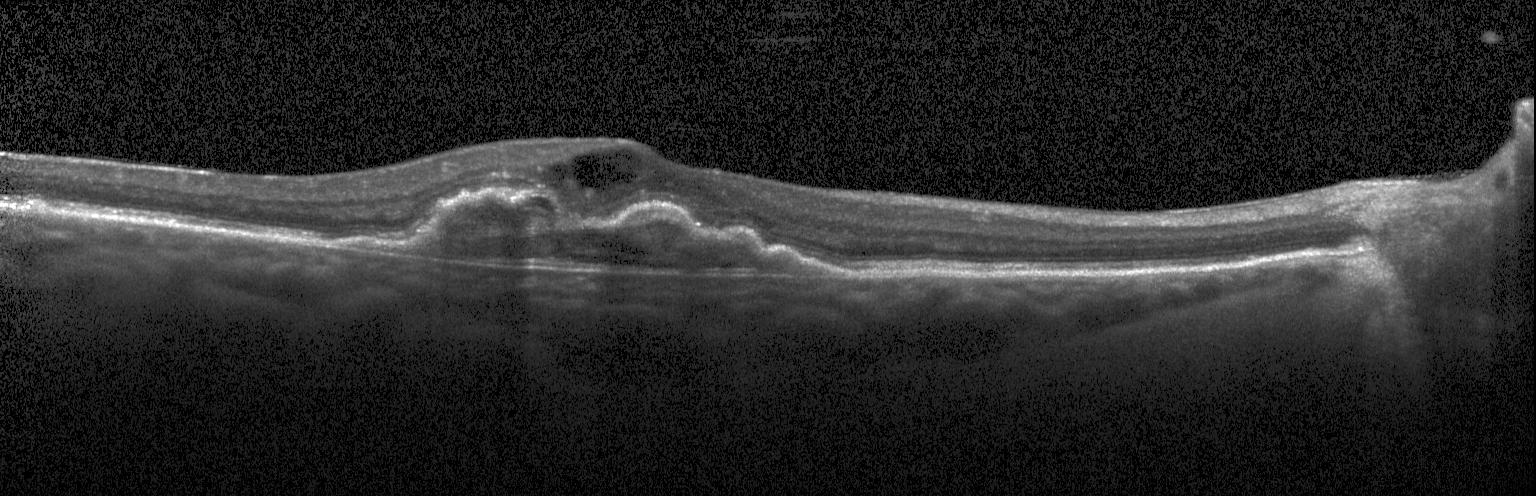
Diagnosis: a choroidal neovascular membrane.